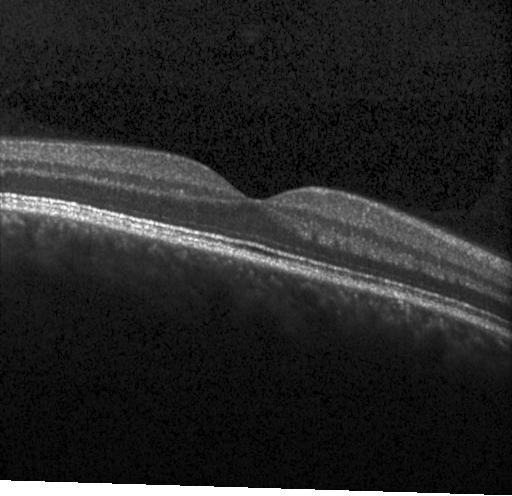

Optical coherence tomography B-scan; instrument: Heidelberg Spectralis; horizontal scan through the fovea; SD-OCT. Finding: neither CNV, DME, nor drusen.